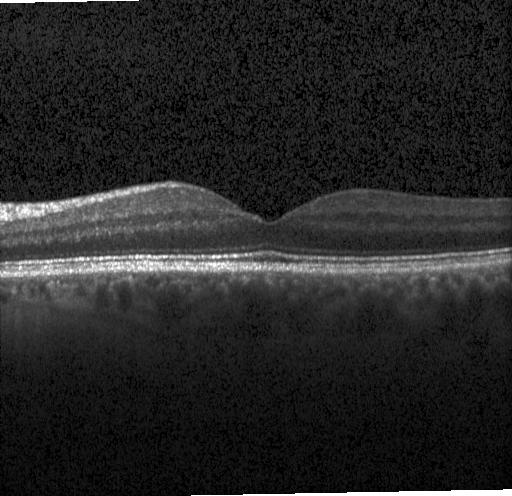 OCT B-scan.
OCT finding: no choroidal neovascularization, no diabetic macular edema, and no drusen.